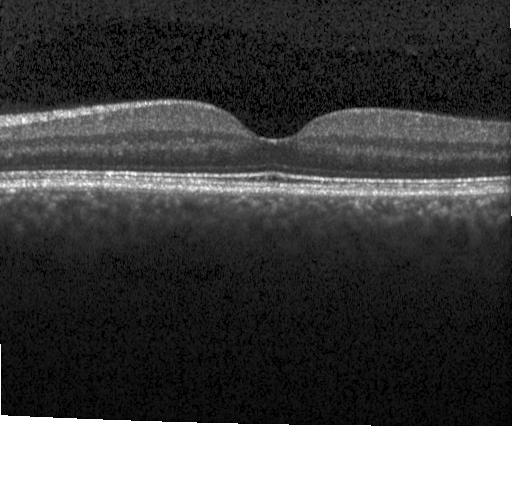

Finding: no choroidal neovascularization, no diabetic macular edema, and no drusen.